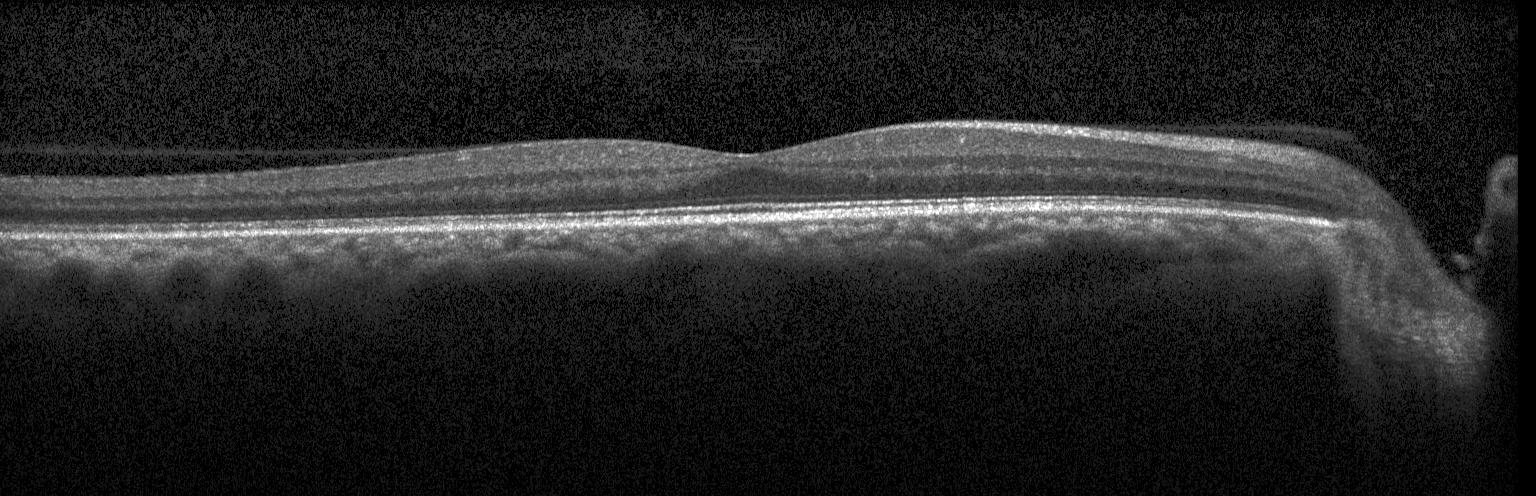
Neither CNV, DME, nor drusen.